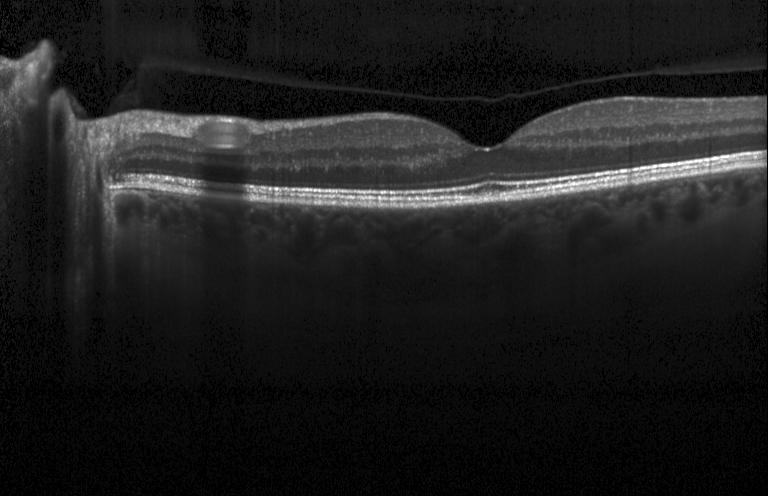

Heidelberg Spectralis; fovea-centered; SD-OCT; optical coherence tomography B-scan — Macular OCT: no choroidal neovascularization, diabetic macular edema, or drusen.